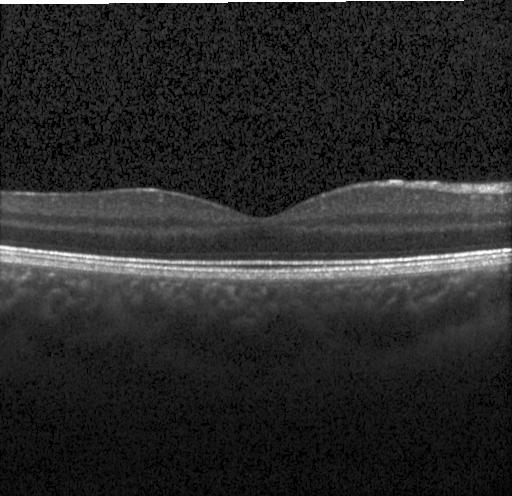
OCT B-scan. Diagnosis: no choroidal neovascularization, no diabetic macular edema, and no drusen.